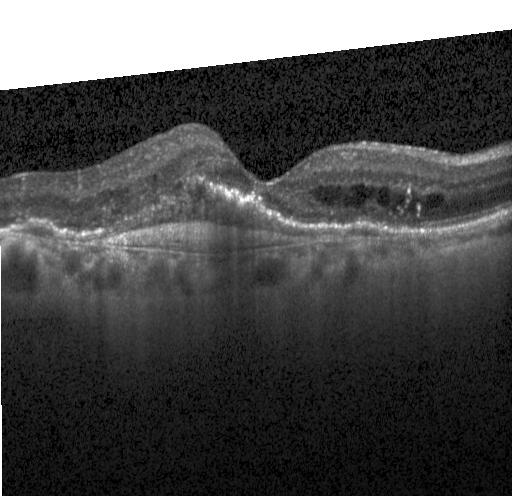

Macular OCT: CNV.